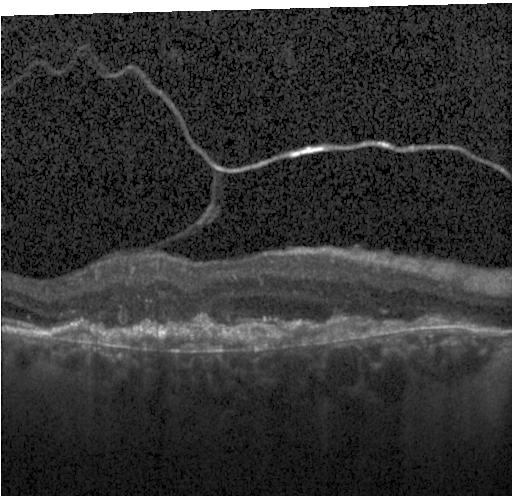 OCT line scan — Macular OCT: choroidal neovascularization (CNV).